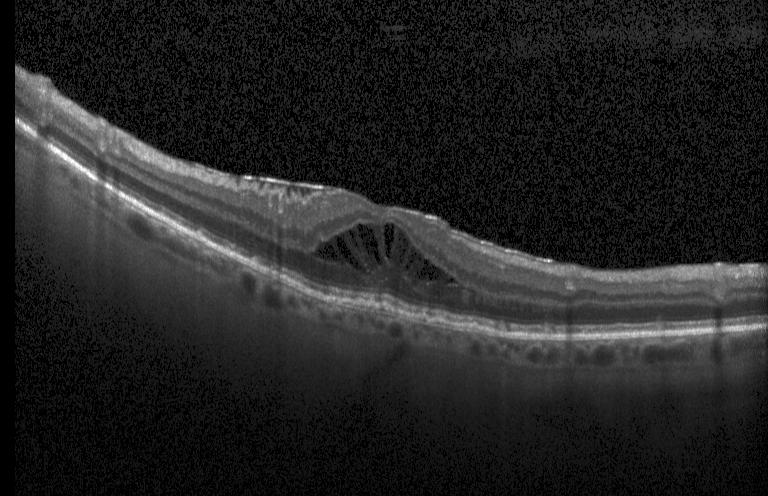
The scan shows diabetic macular edema.